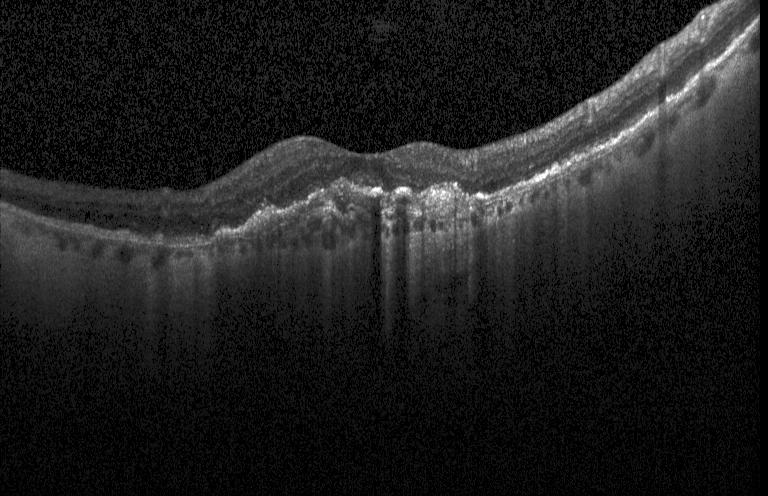 Optical coherence tomography B-scan; Heidelberg Spectralis OCT system.
Choroidal neovascularization (CNV).